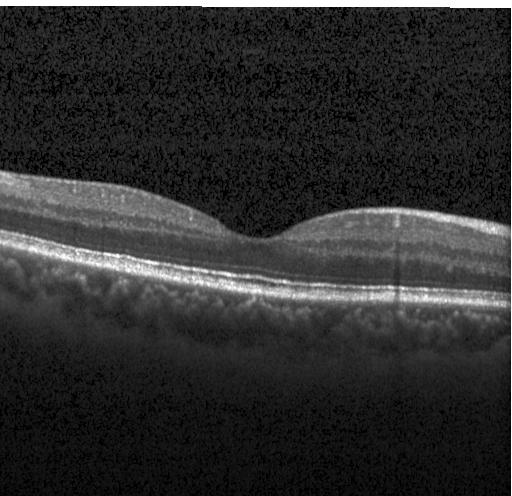

Spectral-domain OCT. OCT B-scan — The scan shows no evidence of choroidal neovascularization, diabetic macular edema, or drusen.